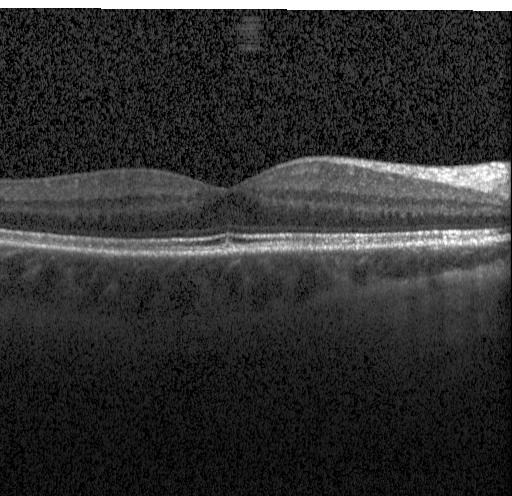
Retinal OCT B-scan · spectral-domain optical coherence tomography — Finding: neither CNV, DME, nor drusen.